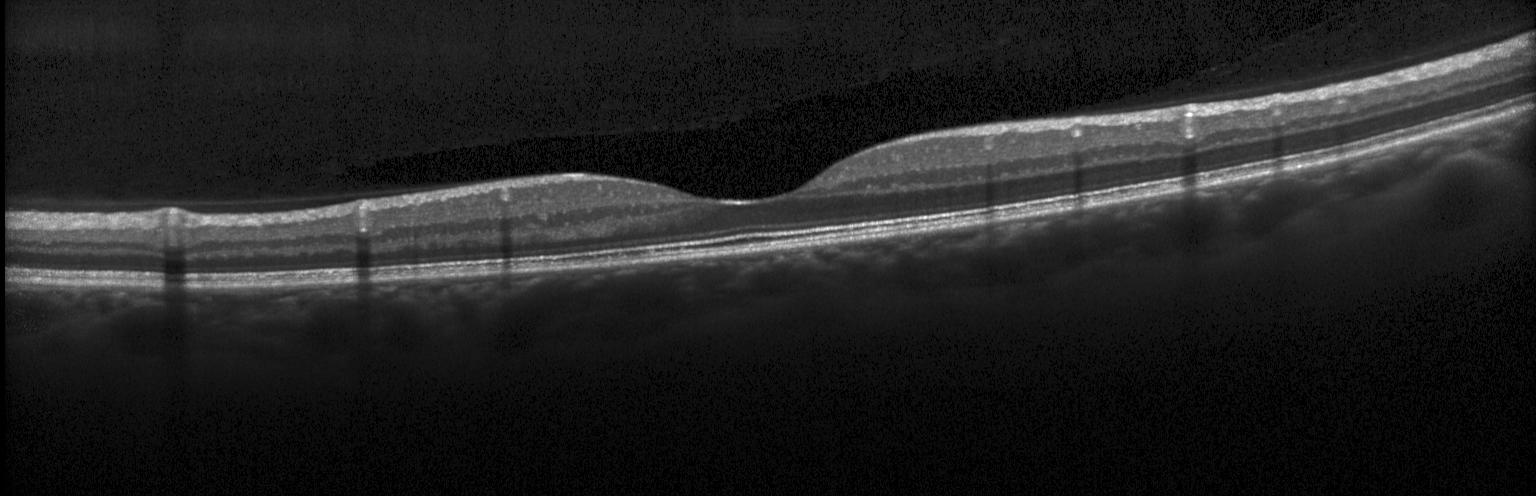 No CNV, no DME, and no drusen.